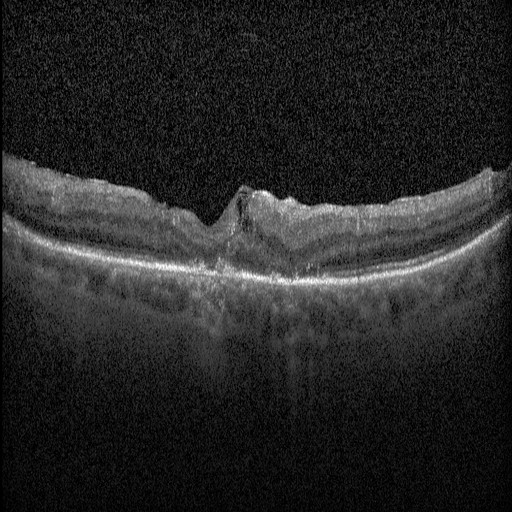 Acquired on a Heidelberg Spectralis; SD-OCT; OCT B-scan; through the macula.
Finding: diabetic macular edema (DME).